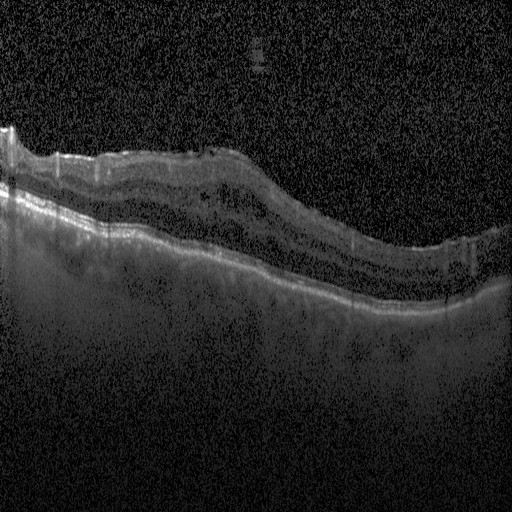

Diabetic macular edema.